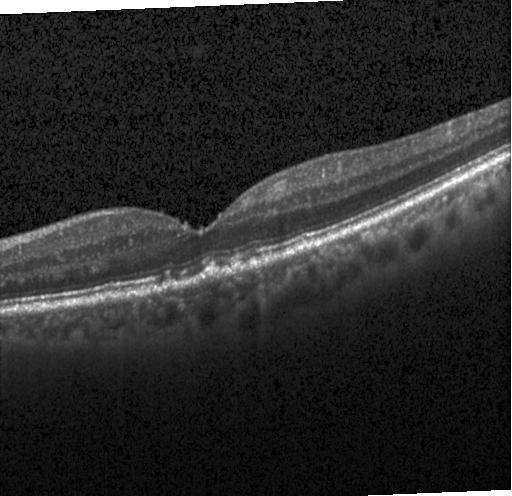

Spectral-domain OCT B-scan: multiple drusen.